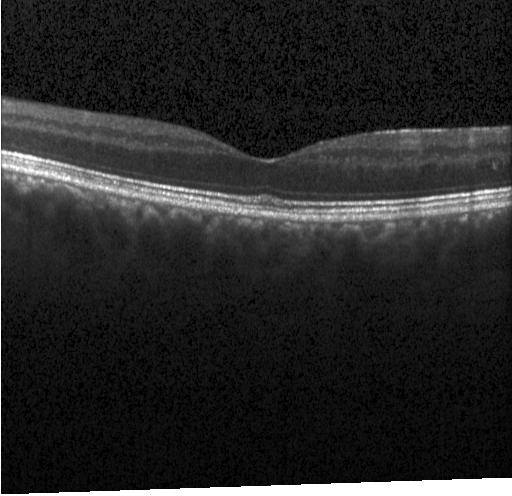
Assessment: no choroidal neovascularization, diabetic macular edema, or drusen.